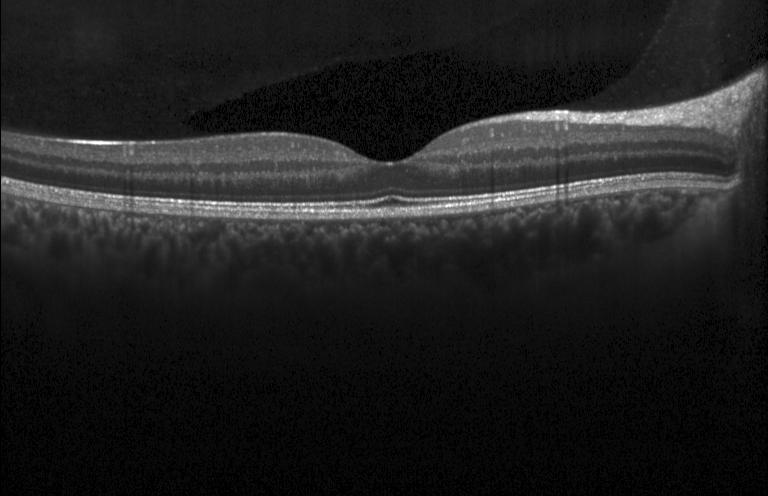 OCT B-scan · horizontal scan through the fovea. Macular OCT: no choroidal neovascularization, diabetic macular edema, or drusen.